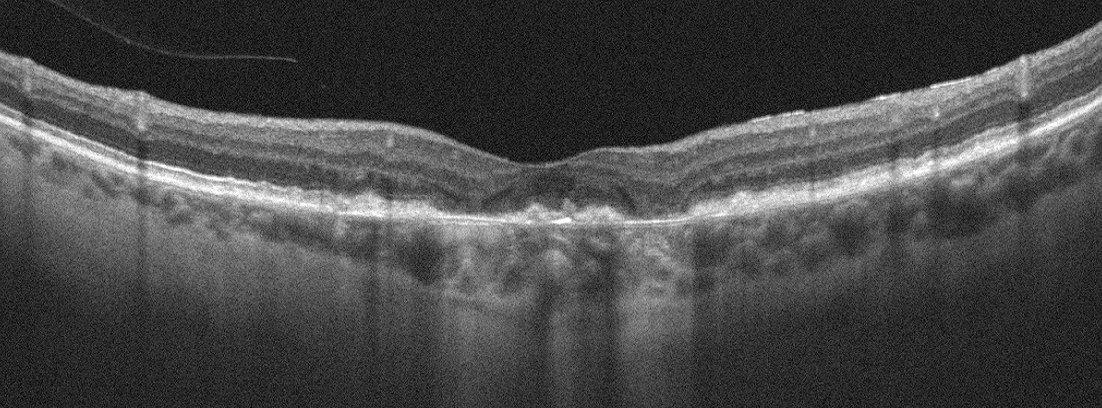

Macular scan. Acquired on an Optovue Avanti RTVue XR. Retinal OCT B-scan — Assessment: age-related macular degeneration.